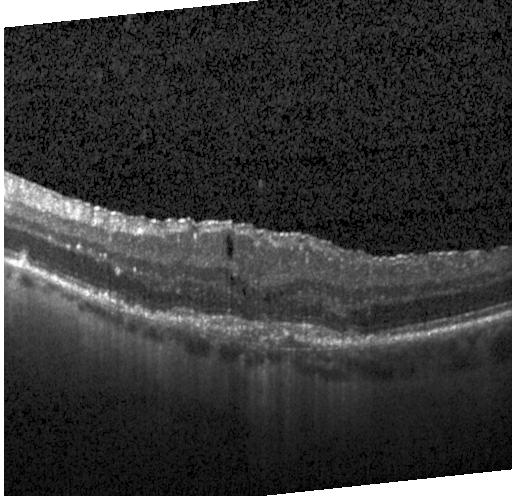

Diagnosis: CNV.